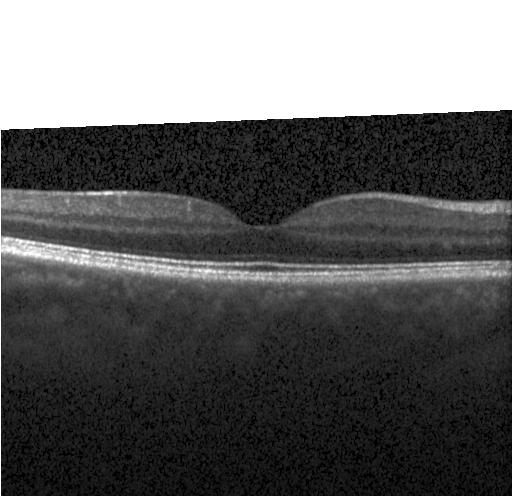
OCT line scan. Finding: no evidence of choroidal neovascularization, diabetic macular edema, or drusen.